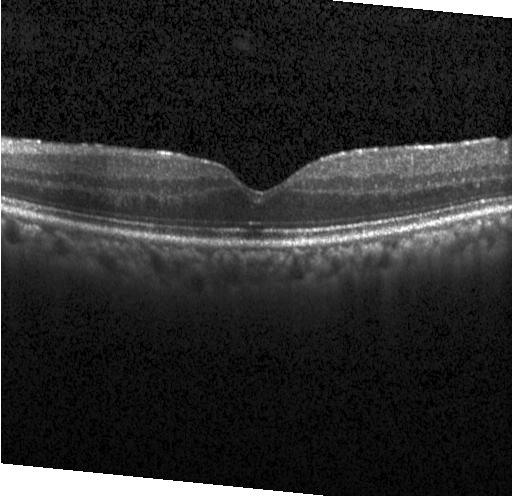 Acquired on a Heidelberg Spectralis · retinal OCT B-scan · horizontal scan through the fovea
Impression: no evidence of choroidal neovascularization, diabetic macular edema, or drusen.